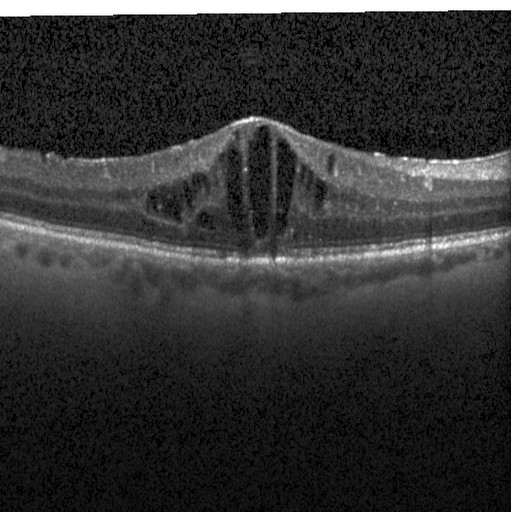

Macular OCT: DME.